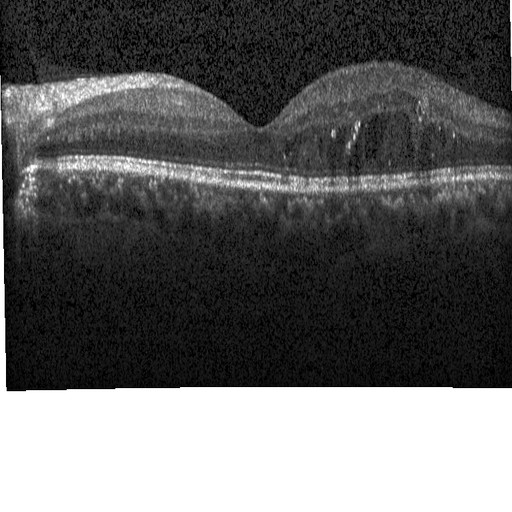 Retinal OCT B-scan. Impression: DME.